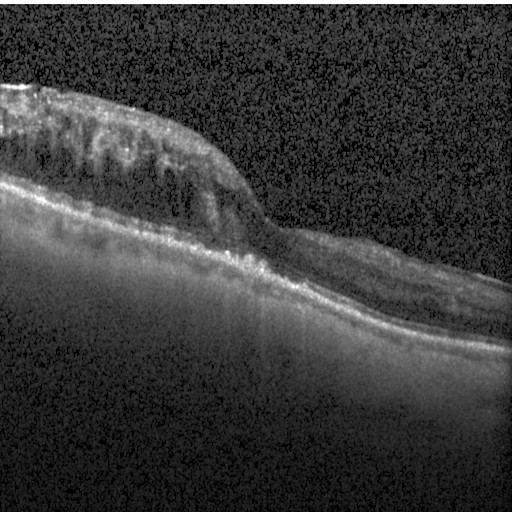 Finding: DME.